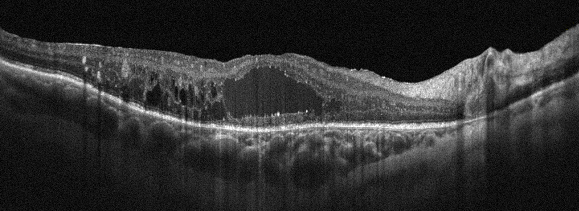

OCT scan showing diabetic macular edema (DME).